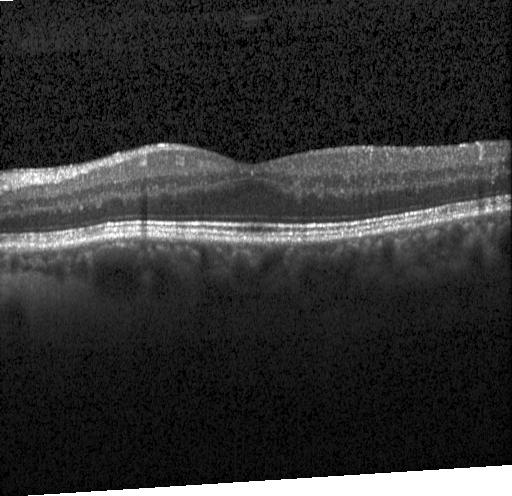 Spectral-domain OCT B-scan: no evidence of choroidal neovascularization, diabetic macular edema, or drusen.